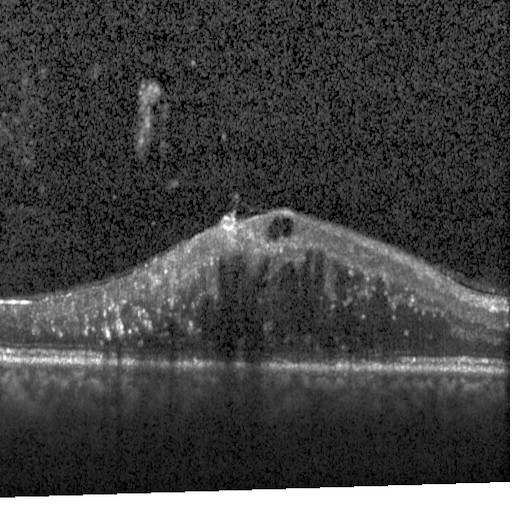

Acquired on a Heidelberg Spectralis; spectral-domain OCT; retinal OCT cross-section — Impression: diabetic macular edema (DME).